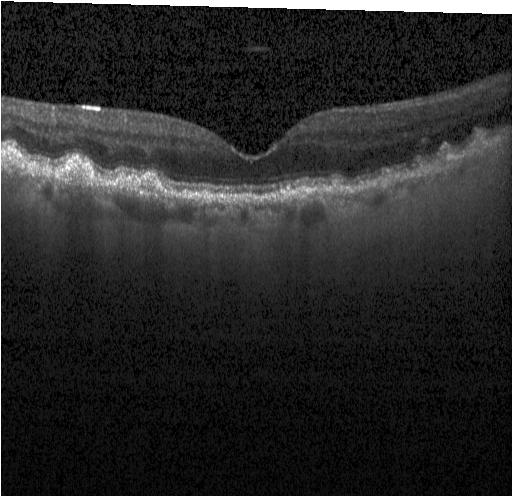 OCT line scan. Assessment: sub-RPE drusenoid deposits.